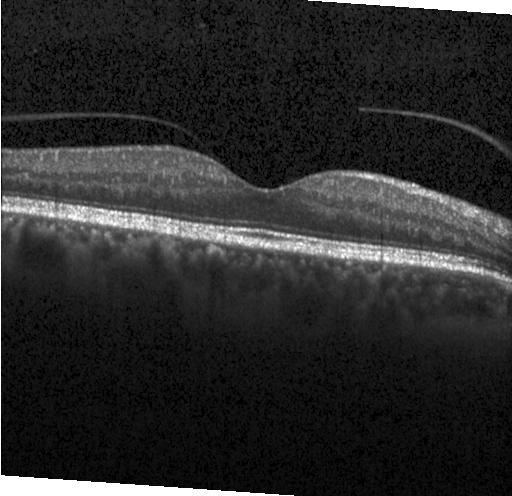

Retinal OCT B-scan.
Dx: no CNV, no DME, and no drusen.